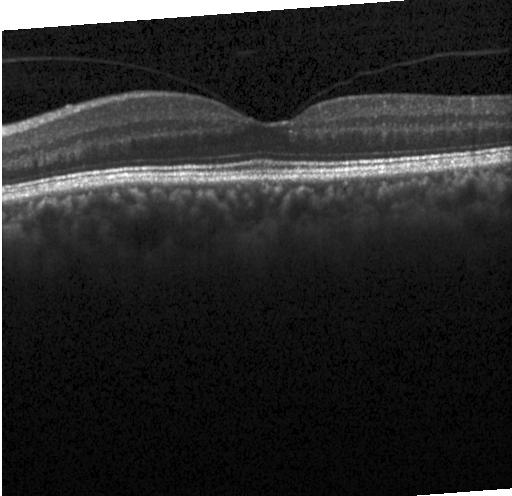
OCT B-scan · Heidelberg Spectralis OCT system · spectral-domain OCT · macular scan. Assessment: no evidence of choroidal neovascularization, diabetic macular edema, or drusen.